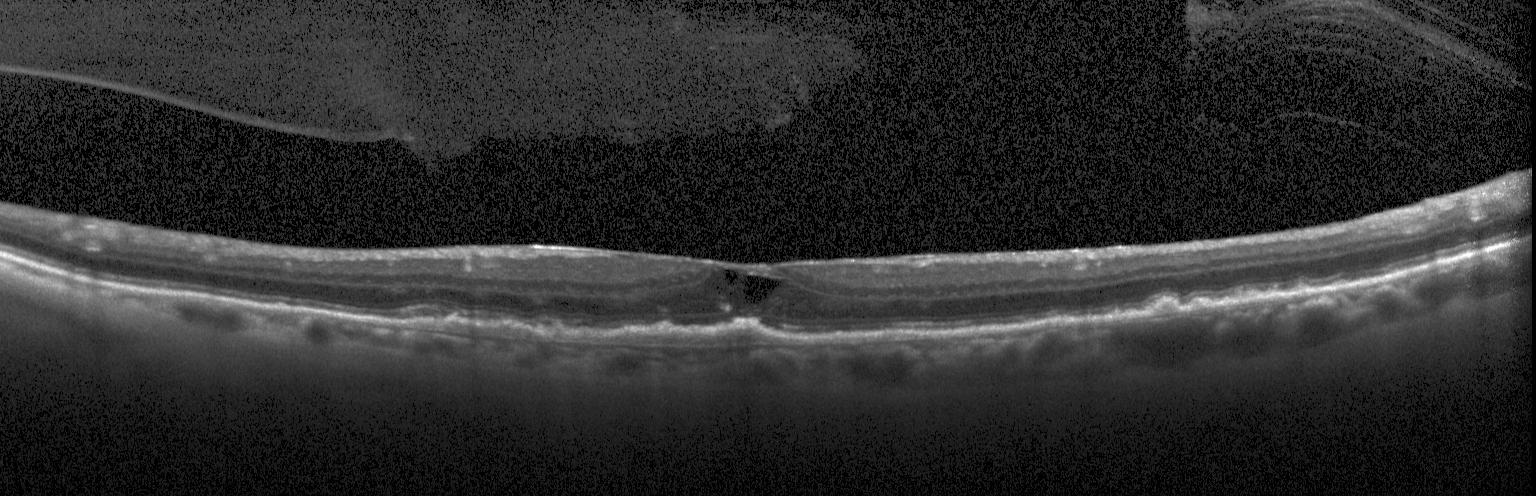
Macular OCT: choroidal neovascularization (CNV).